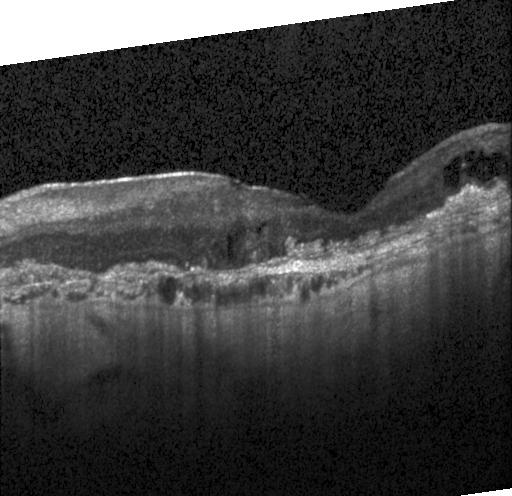 Finding: a choroidal neovascular membrane.